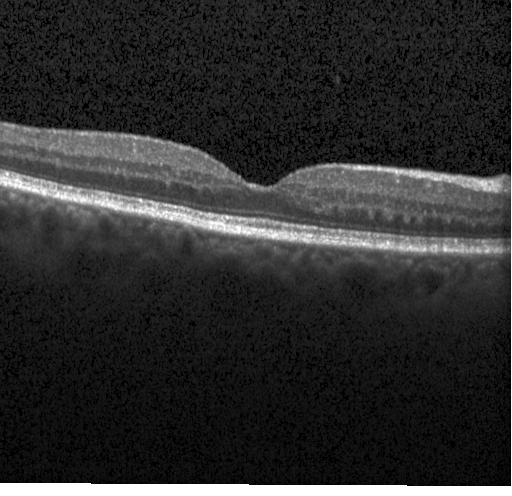

No CNV, no DME, and no drusen.